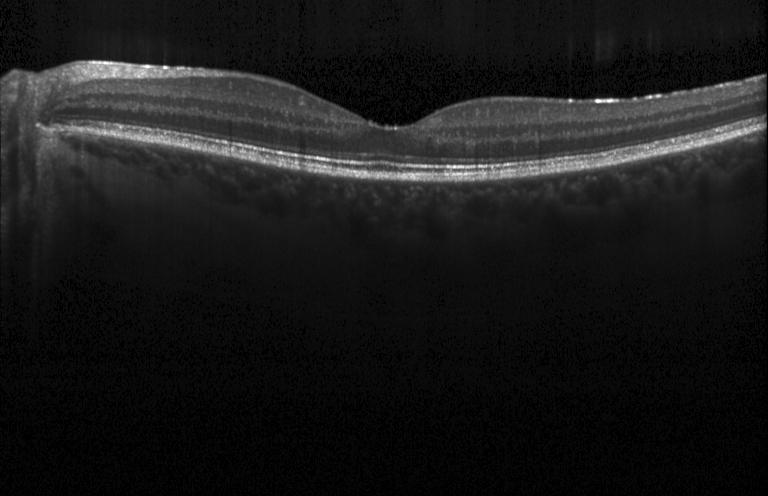
Spectral-domain OCT. Optical coherence tomography B-scan.
Impression: no evidence of choroidal neovascularization, diabetic macular edema, or drusen.